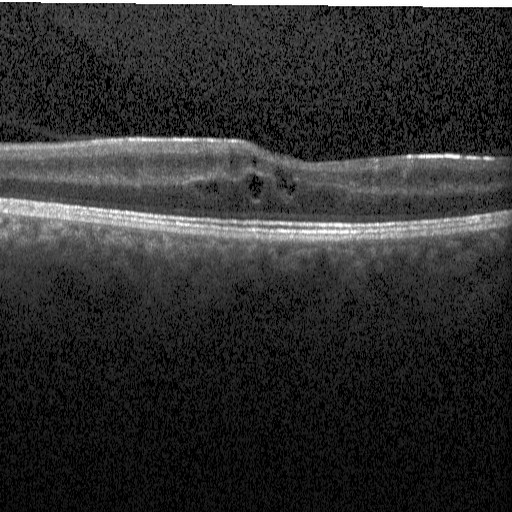 Through the macula, retinal OCT cross-section, spectral-domain OCT.
Macular OCT: DME.